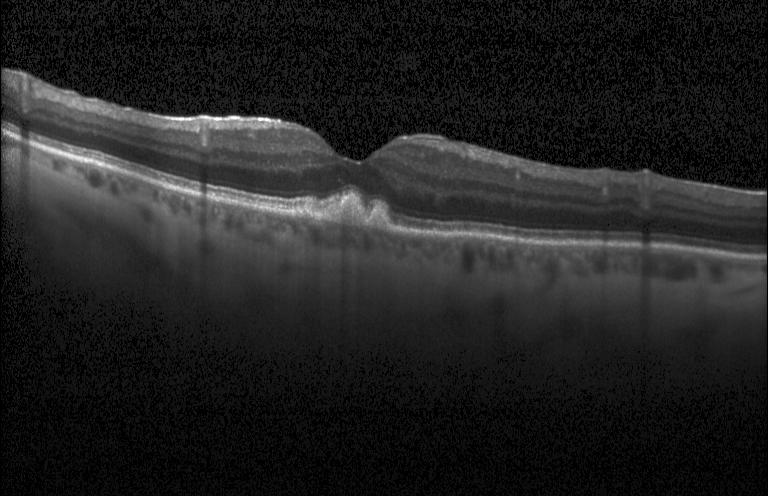
Impression: drusen.